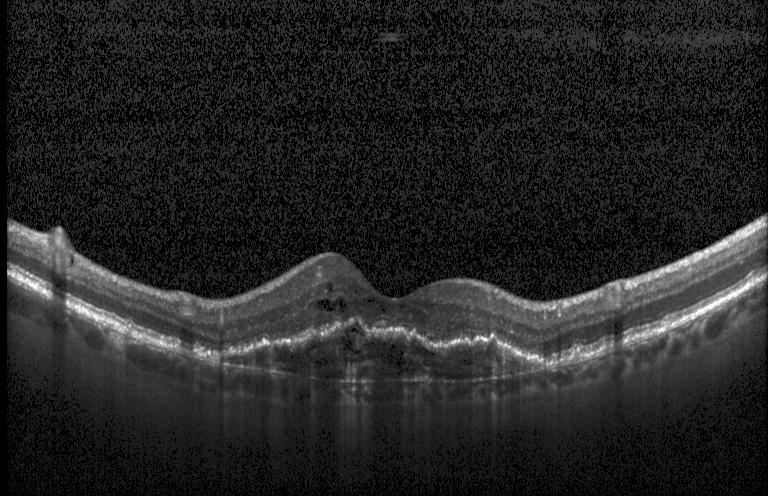 A choroidal neovascular membrane.